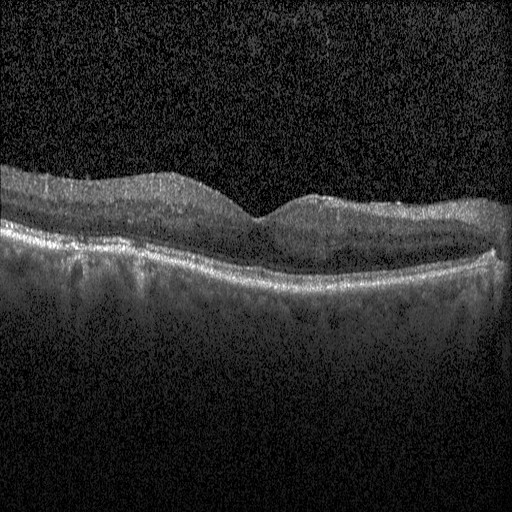
Impression: diabetic macular edema (DME).